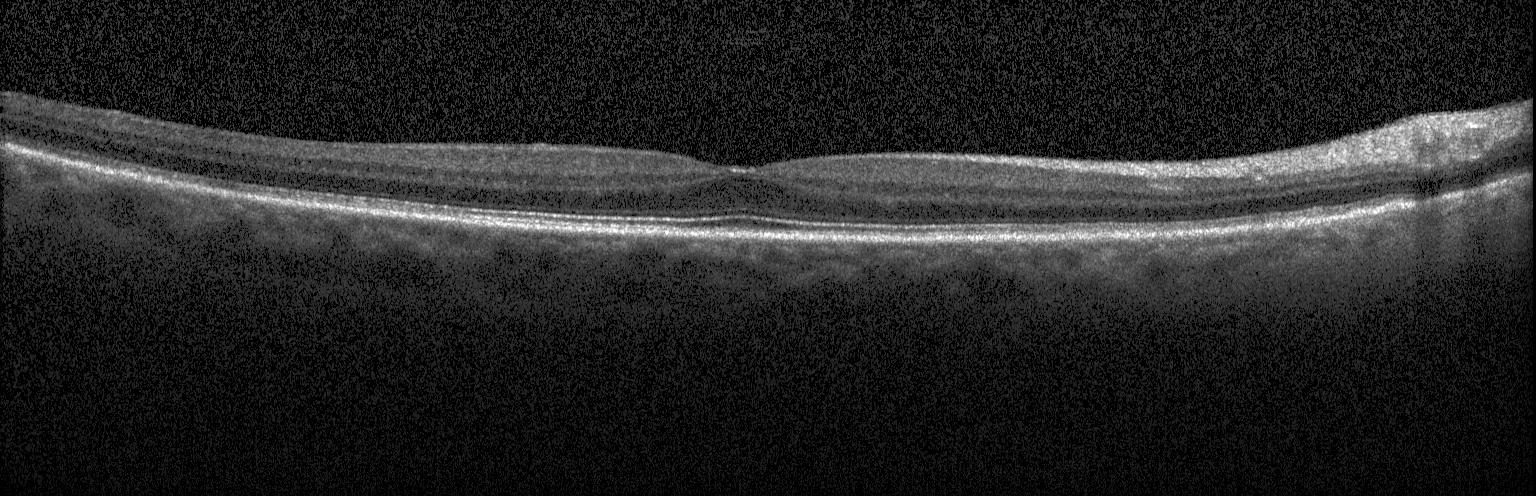

Acquired on a Heidelberg Spectralis; OCT line scan; horizontal scan through the fovea. Finding: no evidence of choroidal neovascularization, diabetic macular edema, or drusen.